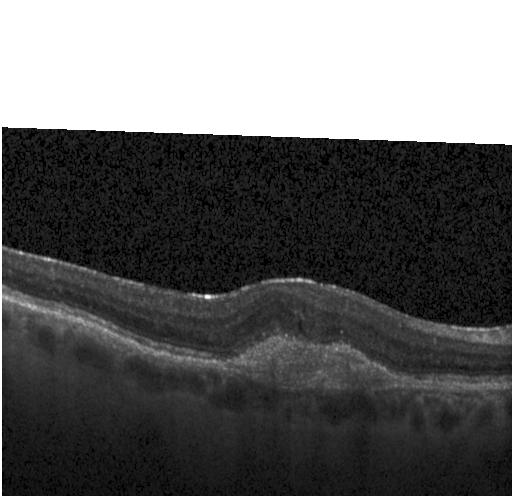

SD-OCT; Heidelberg Spectralis OCT system; optical coherence tomography B-scan; horizontal scan through the fovea. Diagnosis: CNV.